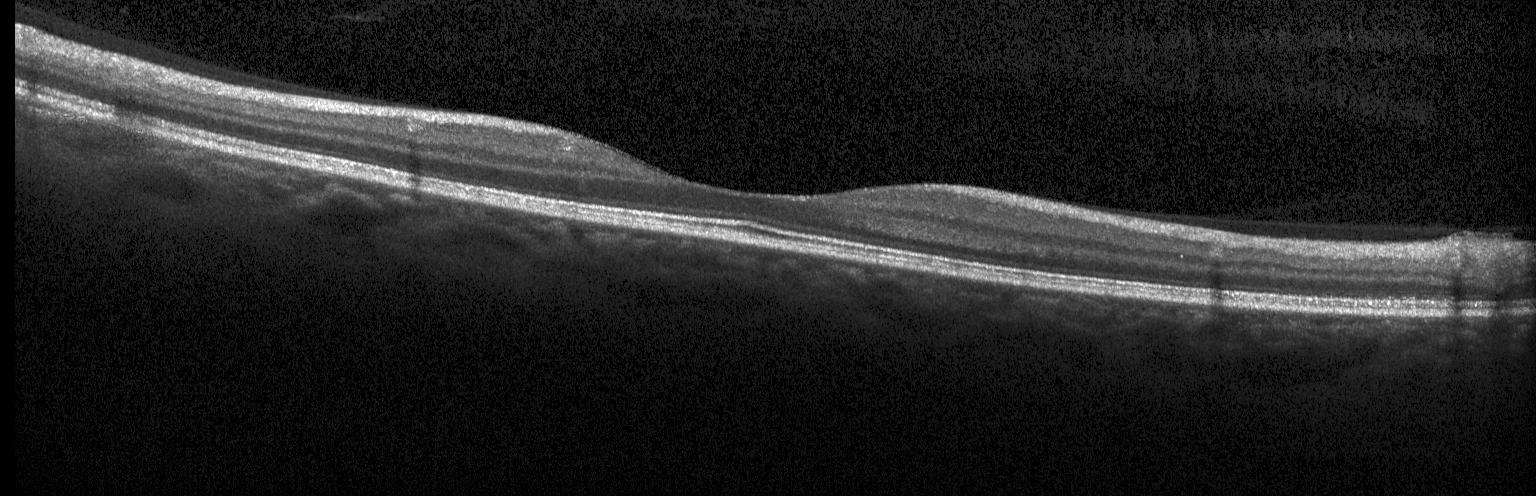
Heidelberg Spectralis OCT system, fovea-centered, optical coherence tomography scan — Finding: neither choroidal neovascularization, diabetic macular edema, nor drusen.